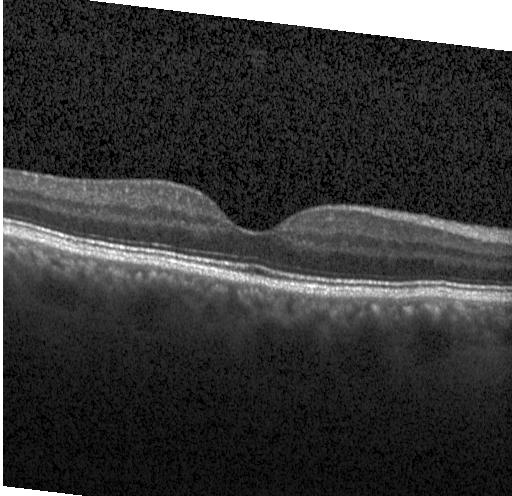

Optical coherence tomography B-scan. Impression: no choroidal neovascularization, diabetic macular edema, or drusen.